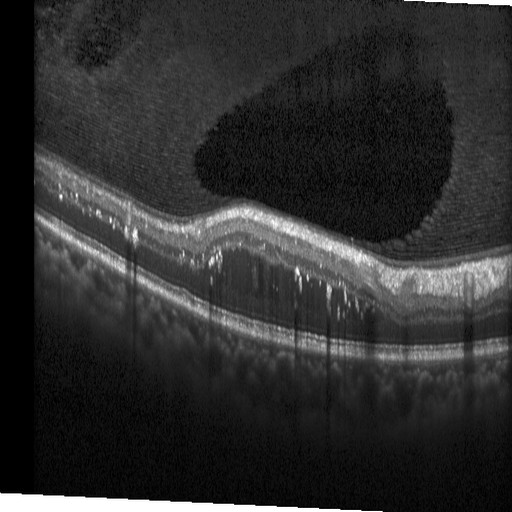 Macular OCT: DME.